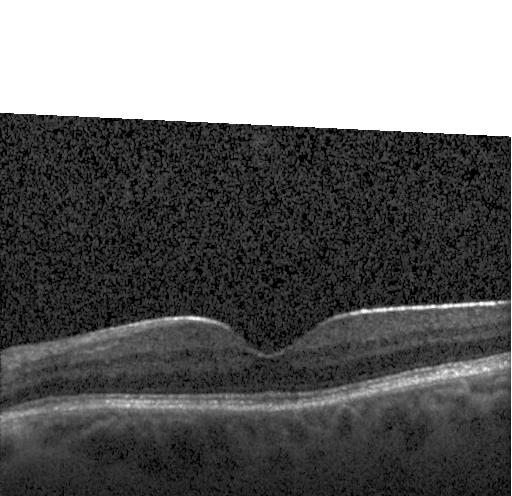 Retinal OCT cross-section; acquired on a Heidelberg Spectralis; fovea-centered — OCT finding: no CNV, no DME, and no drusen.